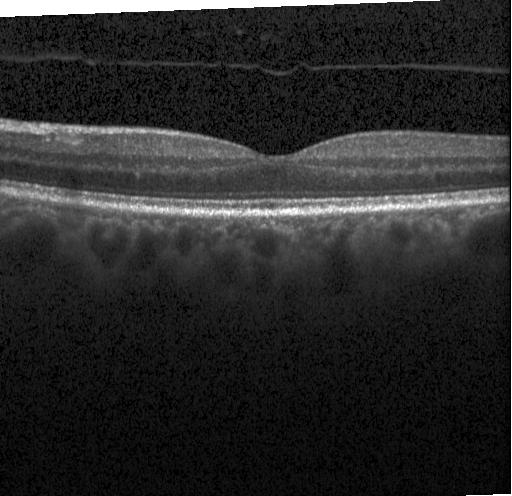

Spectral-domain OCT B-scan: no choroidal neovascularization, no diabetic macular edema, and no drusen.